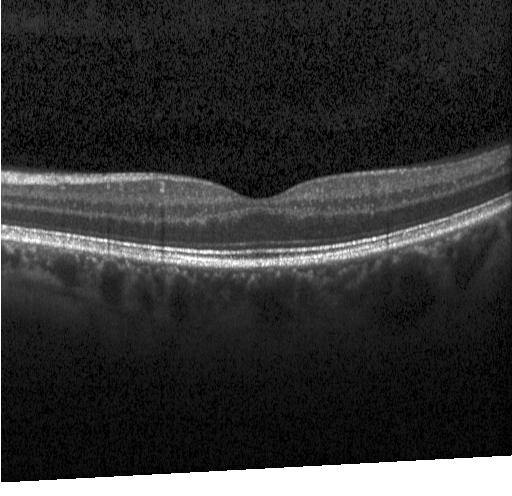 SD-OCT · OCT line scan. Diagnosis: no evidence of choroidal neovascularization, diabetic macular edema, or drusen.